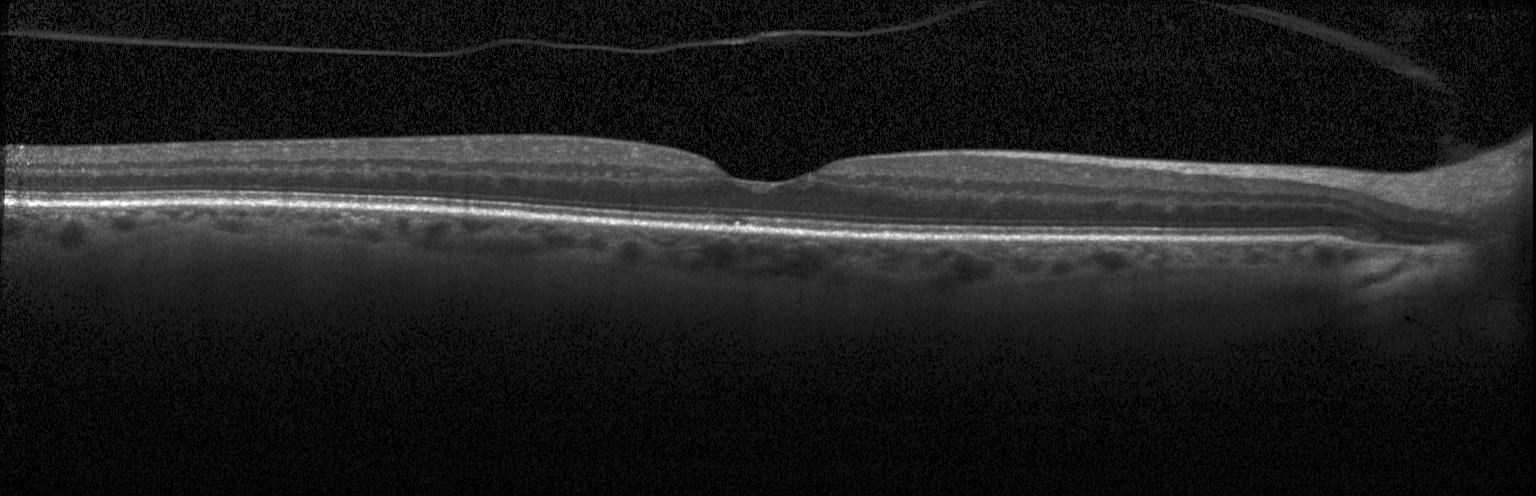 This B-scan demonstrates no choroidal neovascularization, diabetic macular edema, or drusen.